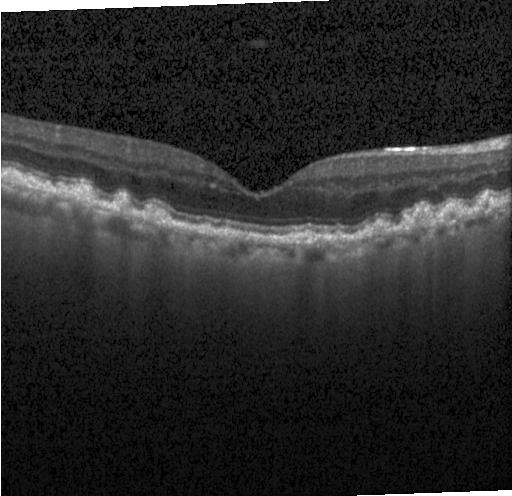

Impression: sub-RPE drusenoid deposits.